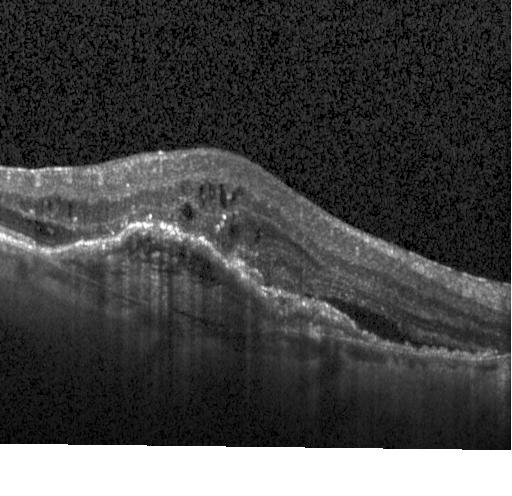

Assessment: a choroidal neovascular membrane.